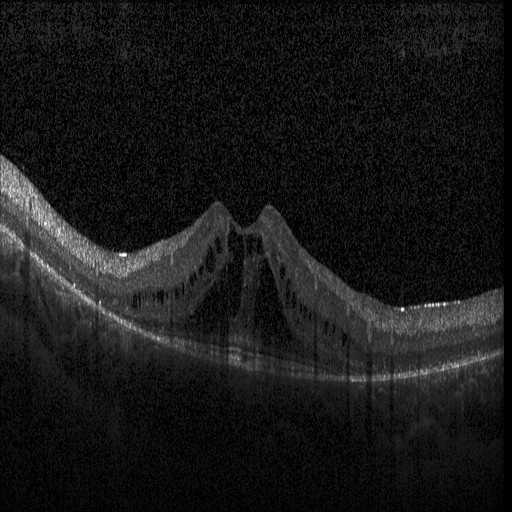
Retinal OCT B-scan · SD-OCT · fovea-centered — Impression: diabetic macular edema.